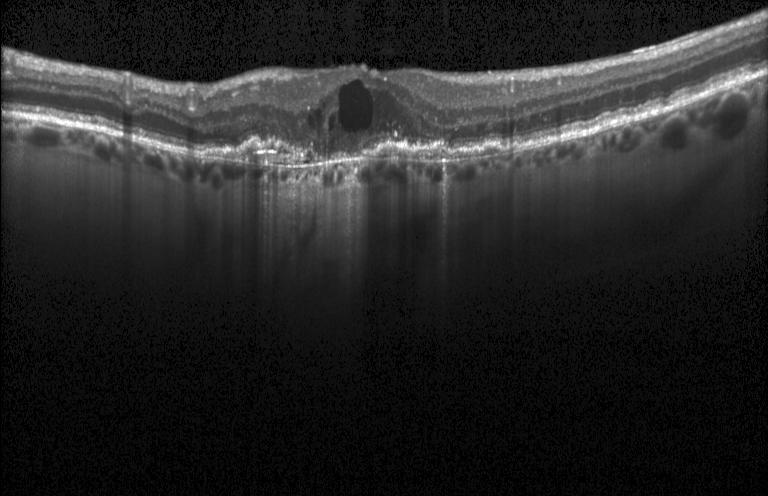 Horizontal scan through the fovea, optical coherence tomography B-scan, spectral-domain optical coherence tomography — Dx: a choroidal neovascular membrane.